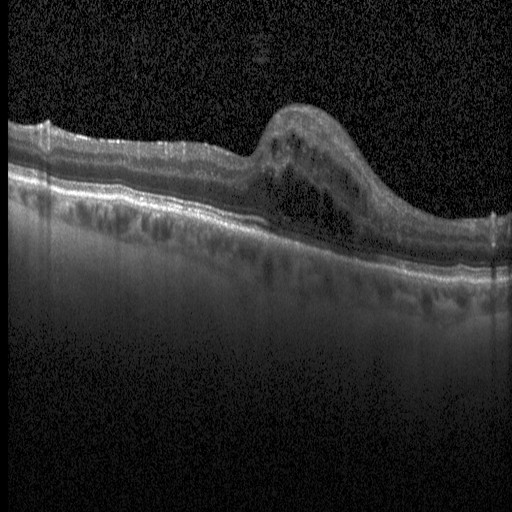

Optical coherence tomography B-scan
Diagnosis: diabetic macular edema (DME).